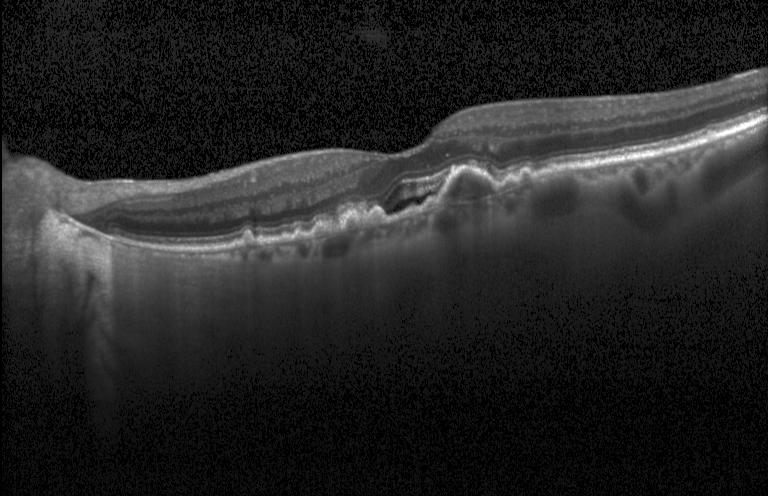
Retinal OCT B-scan, horizontal scan through the fovea, instrument: Heidelberg Spectralis — Macular OCT: a choroidal neovascular membrane.